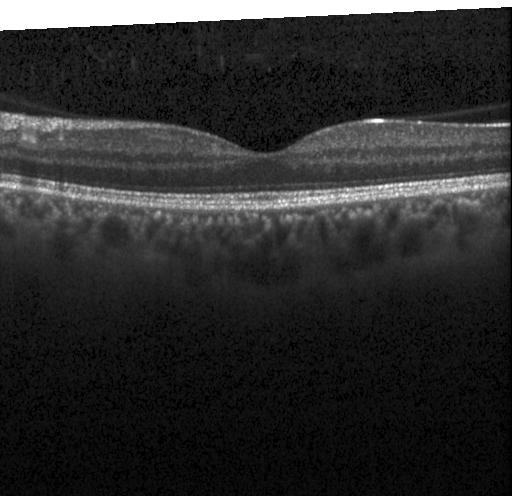
Diagnosis: neither choroidal neovascularization, diabetic macular edema, nor drusen.